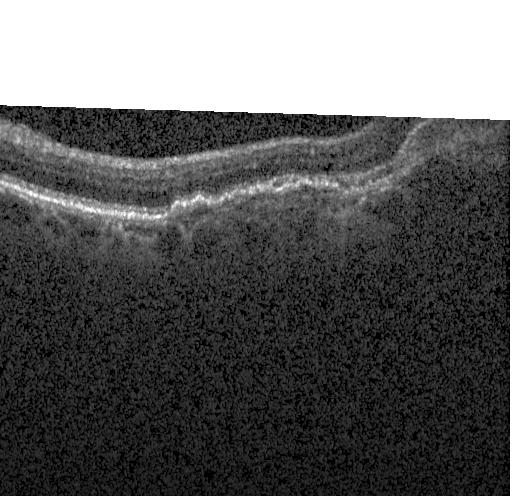
OCT finding: a choroidal neovascular membrane.